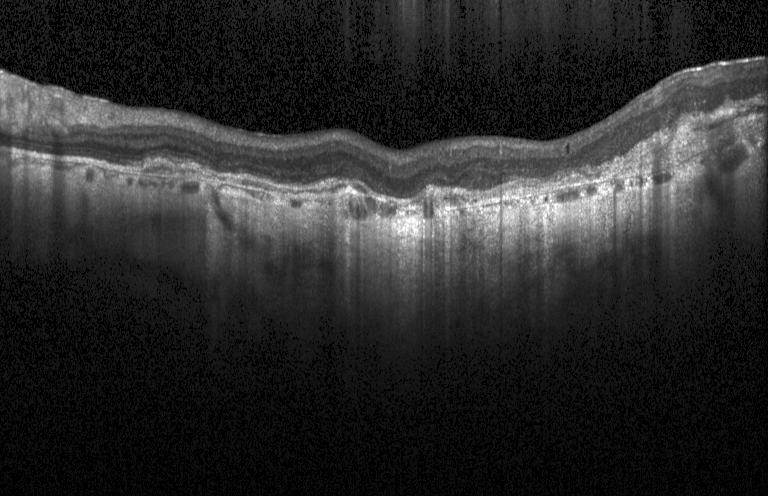
A choroidal neovascular membrane.